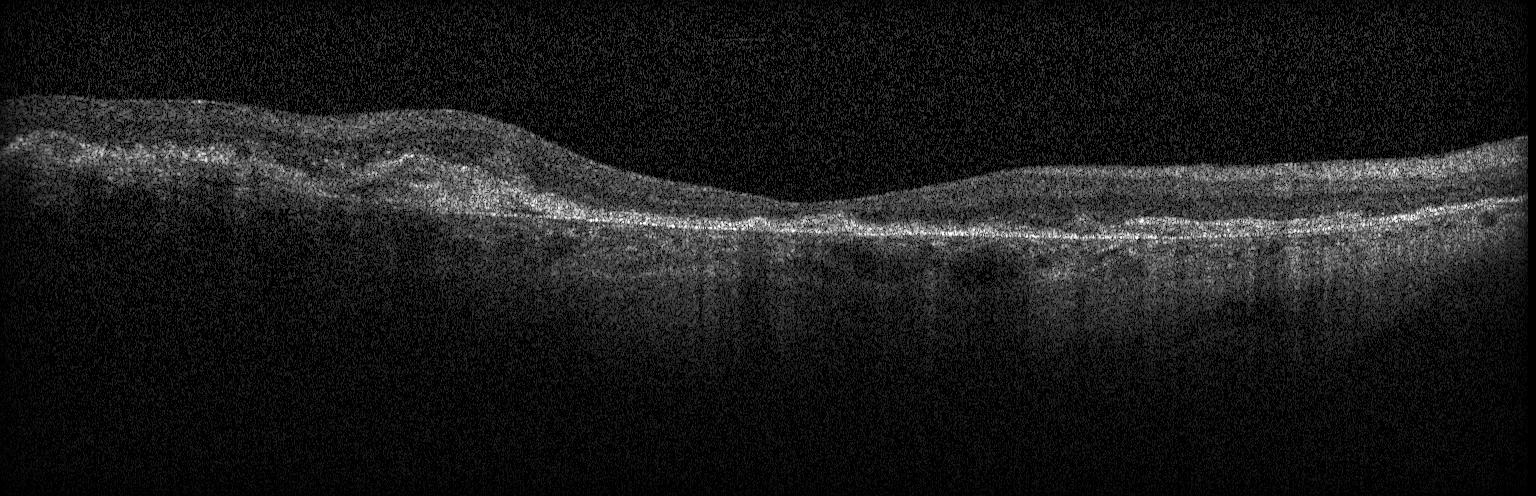 A choroidal neovascular membrane.